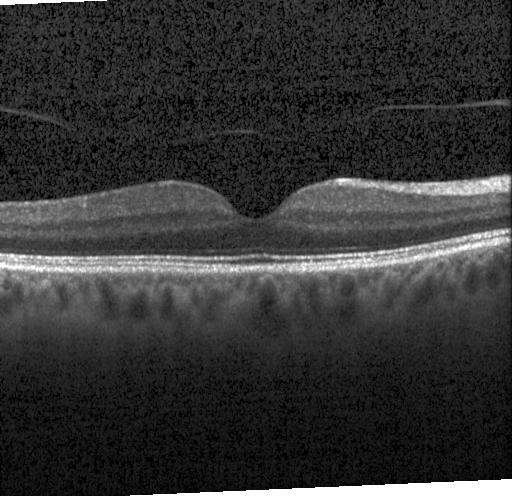
Centered on the fovea · acquired on a Heidelberg Spectralis · OCT line scan.
Dx: no choroidal neovascularization, diabetic macular edema, or drusen.